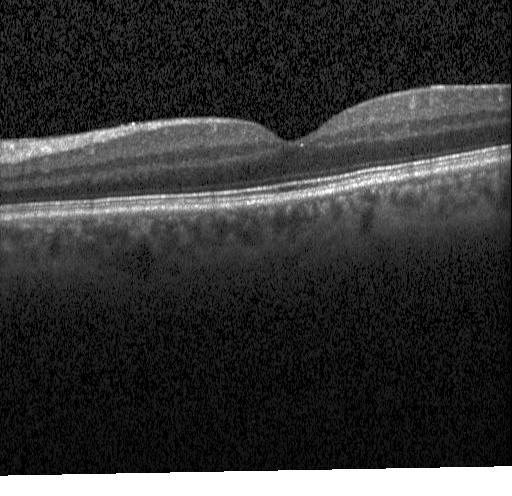
Macular scan; optical coherence tomography B-scan
This B-scan demonstrates neither choroidal neovascularization, diabetic macular edema, nor drusen.